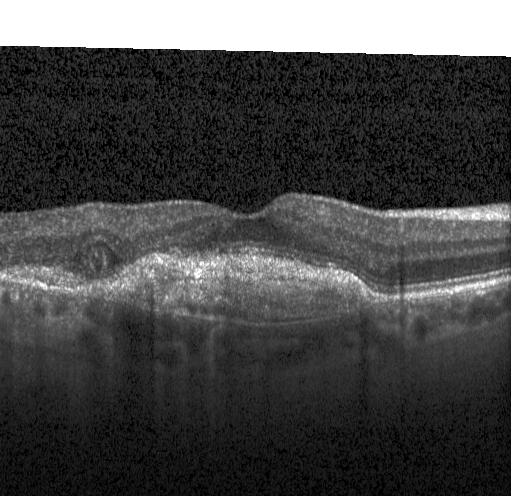
Retinal OCT cross-section showing a choroidal neovascular membrane.